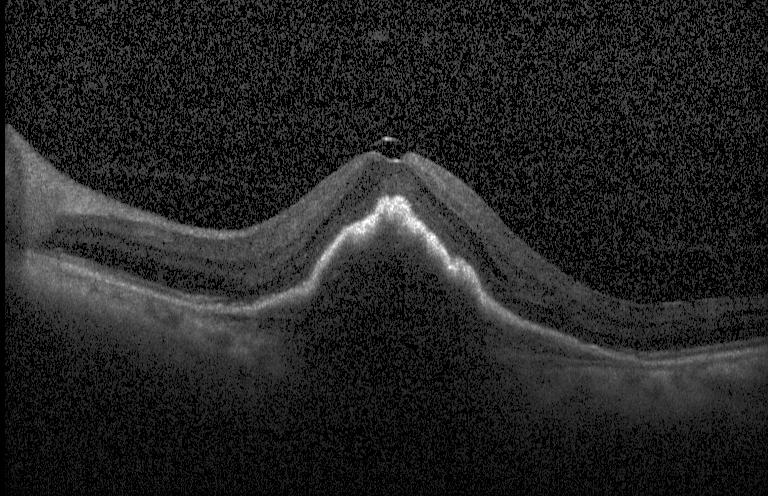
Impression: a choroidal neovascular membrane.